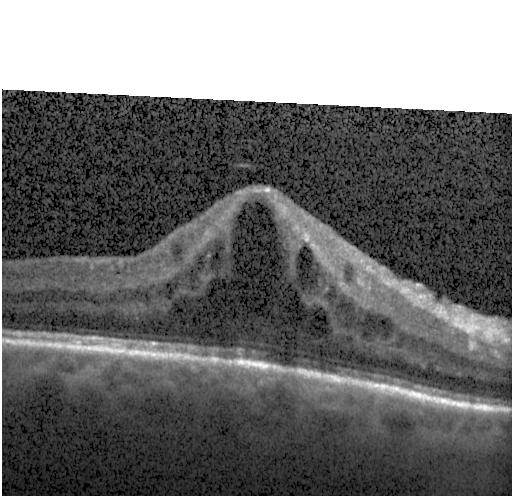 Acquired on a Heidelberg Spectralis; SD-OCT; horizontal scan through the fovea; OCT line scan.
Impression: DME.